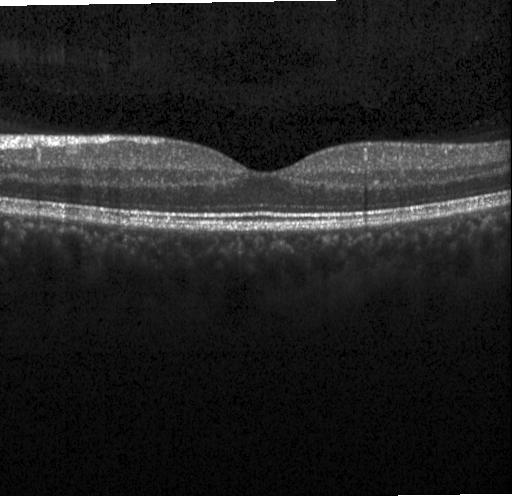
OCT B-scan showing neither choroidal neovascularization, diabetic macular edema, nor drusen.